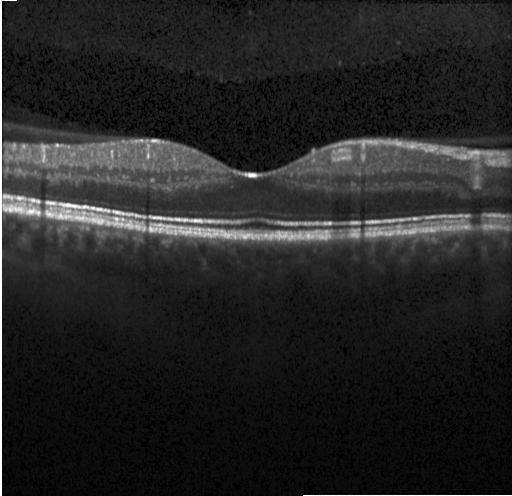
OCT B-scan. Through the macula. SD-OCT.
Finding: neither choroidal neovascularization, diabetic macular edema, nor drusen.